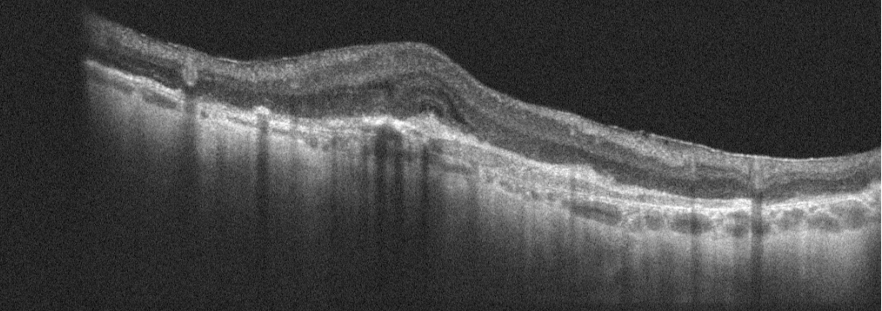 Fovea-centered, optical coherence tomography scan. Impression: age-related macular degeneration (AMD).